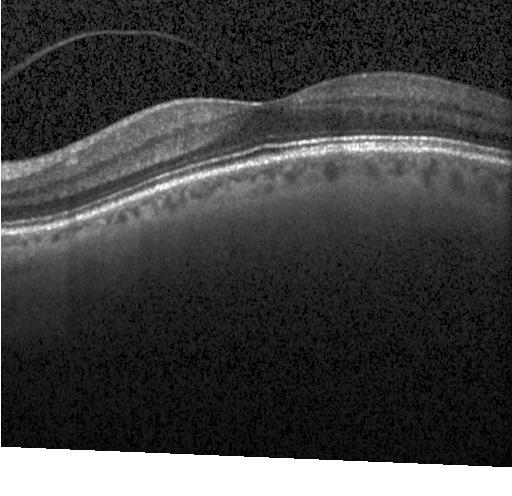

Optical coherence tomography B-scan. No evidence of choroidal neovascularization, diabetic macular edema, or drusen.